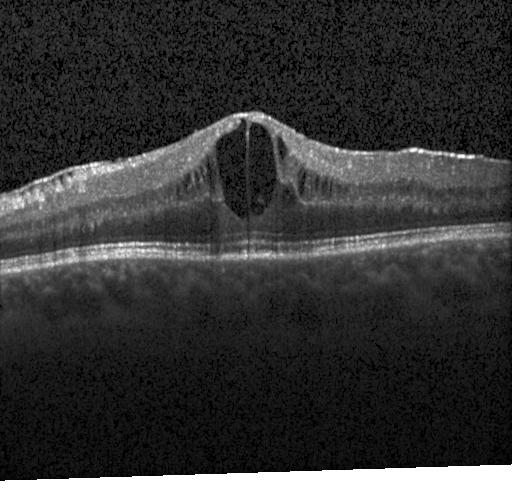 Horizontal scan through the fovea · OCT line scan · Heidelberg Spectralis — Finding: diabetic macular edema.